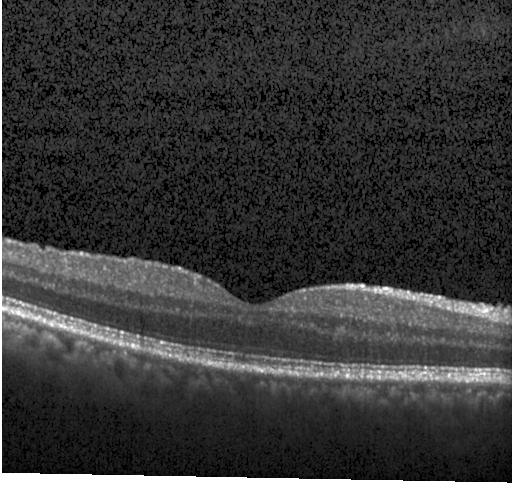
Assessment: no evidence of choroidal neovascularization, diabetic macular edema, or drusen.